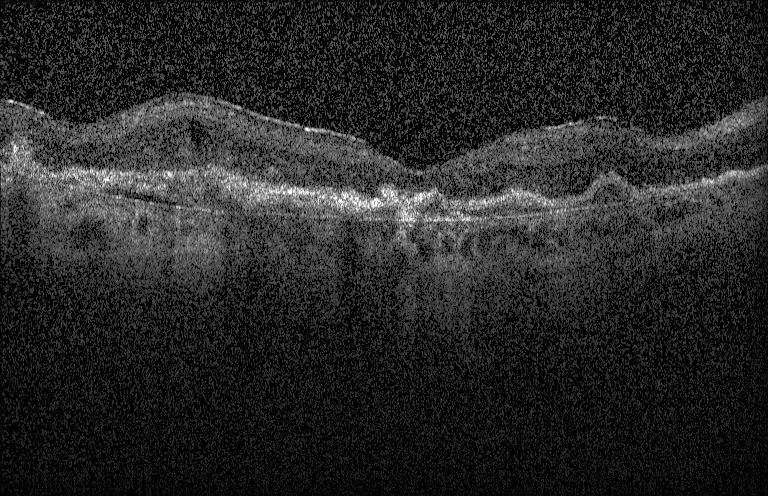
Spectral-domain OCT B-scan: choroidal neovascularization (CNV).